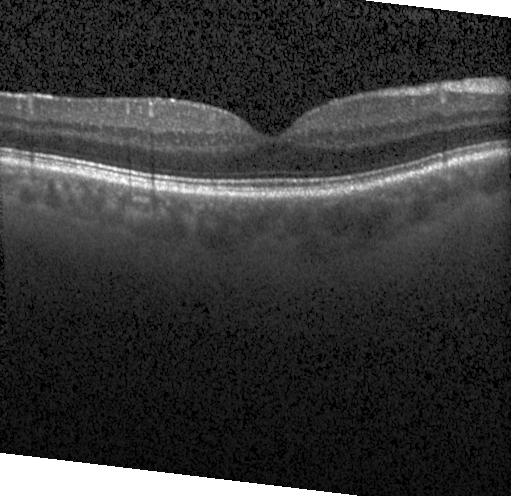
Acquired on a Heidelberg Spectralis · OCT line scan — Diagnosis: no CNV, DME, or drusen.